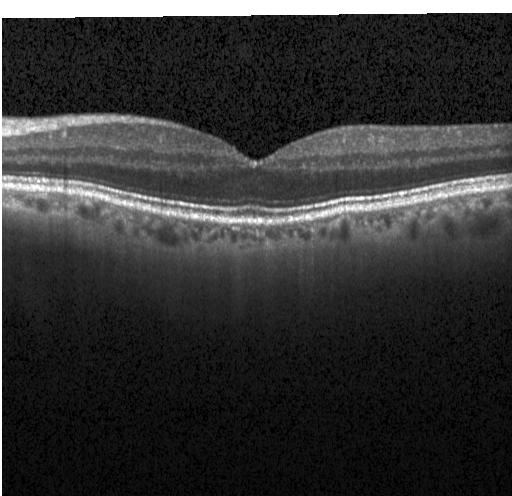 Horizontal scan through the fovea · spectral-domain optical coherence tomography · optical coherence tomography B-scan. Finding: neither choroidal neovascularization, diabetic macular edema, nor drusen.